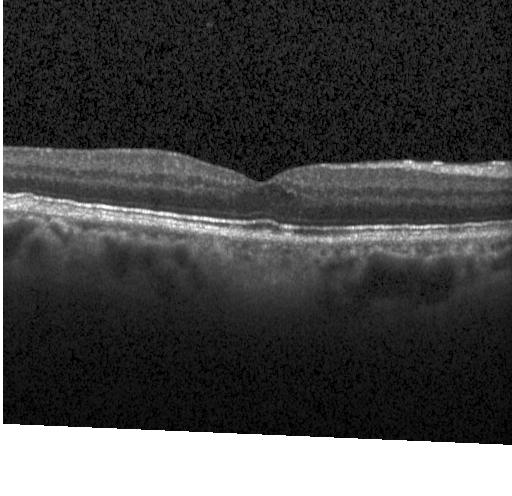
Optical coherence tomography B-scan.
Finding: no CNV, no DME, and no drusen.